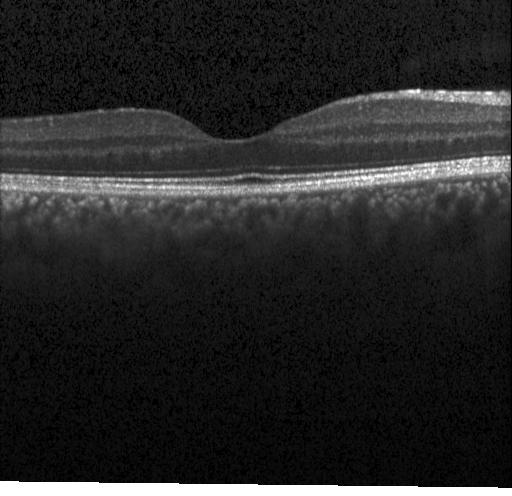 Retinal OCT B-scan
Finding: no choroidal neovascularization, no diabetic macular edema, and no drusen.